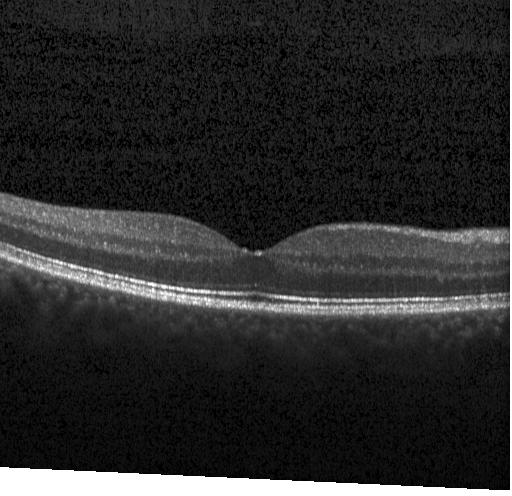

Finding: no CNV, no DME, and no drusen.